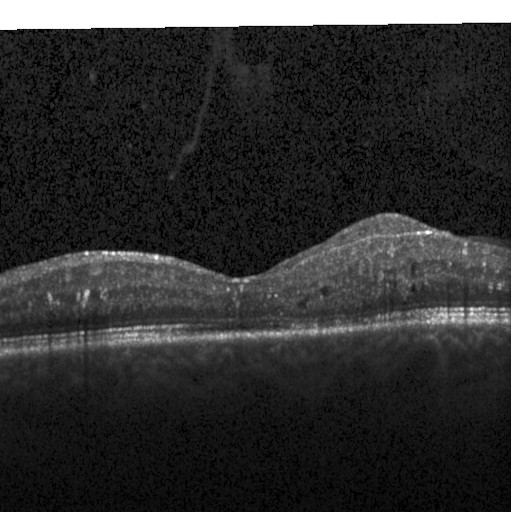

OCT scan showing diabetic macular edema.